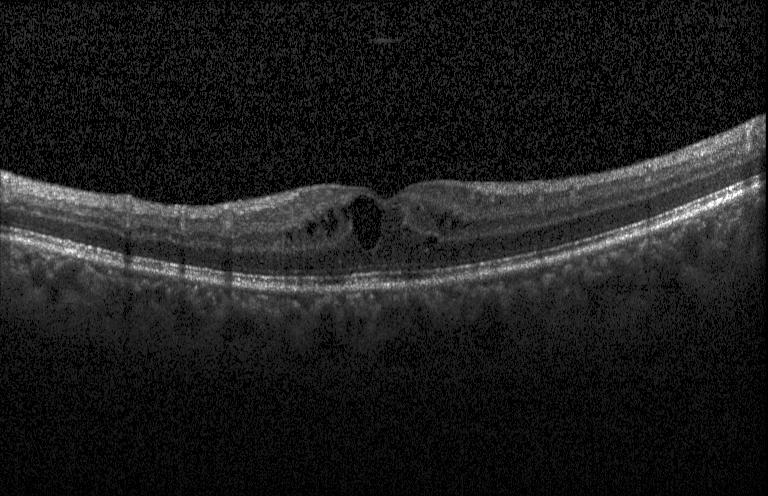 OCT finding: diabetic macular edema.